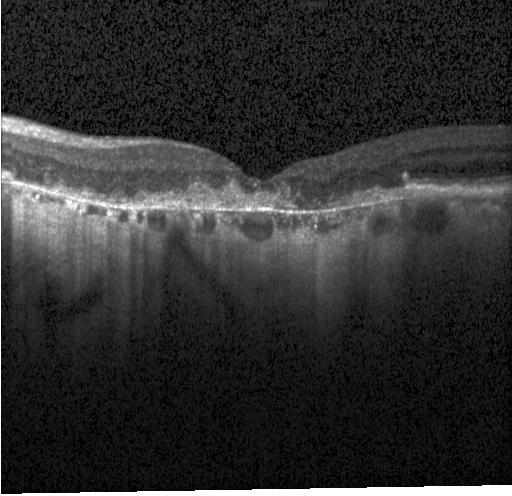 Instrument: Heidelberg Spectralis, optical coherence tomography B-scan, through the macula
Finding: choroidal neovascularization.